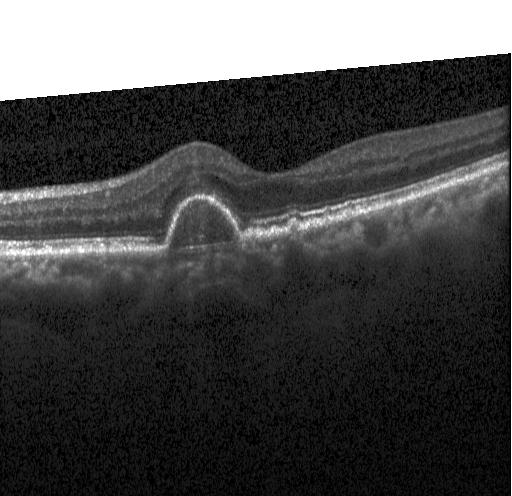
Instrument: Heidelberg Spectralis. Horizontal scan through the fovea. Spectral-domain optical coherence tomography. Retinal OCT cross-section.
OCT finding: drusen.